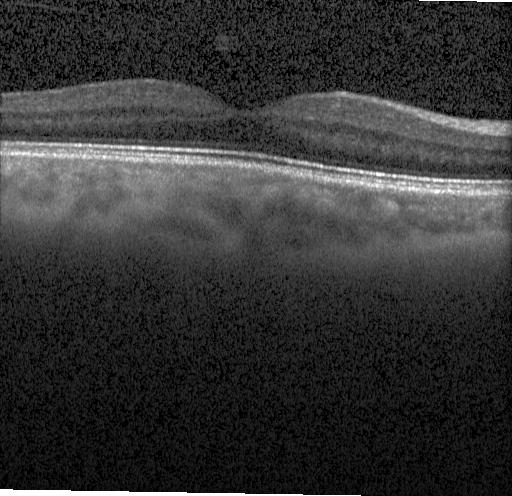 Impression: no CNV, DME, or drusen.